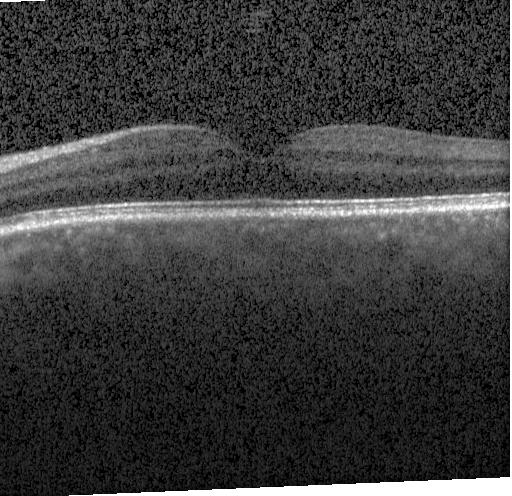
Optical coherence tomography B-scan
Diagnosis: no CNV, DME, or drusen.